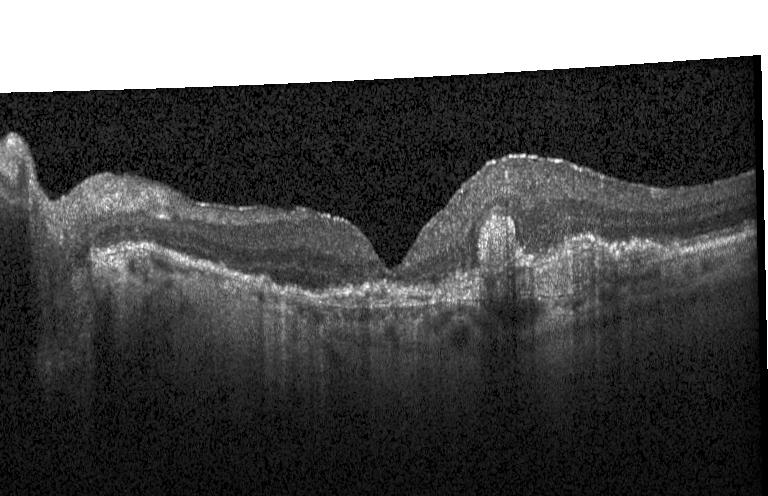

Spectral-domain optical coherence tomography. Fovea-centered. Heidelberg Spectralis OCT system. Optical coherence tomography scan.
OCT finding: choroidal neovascularization (CNV).